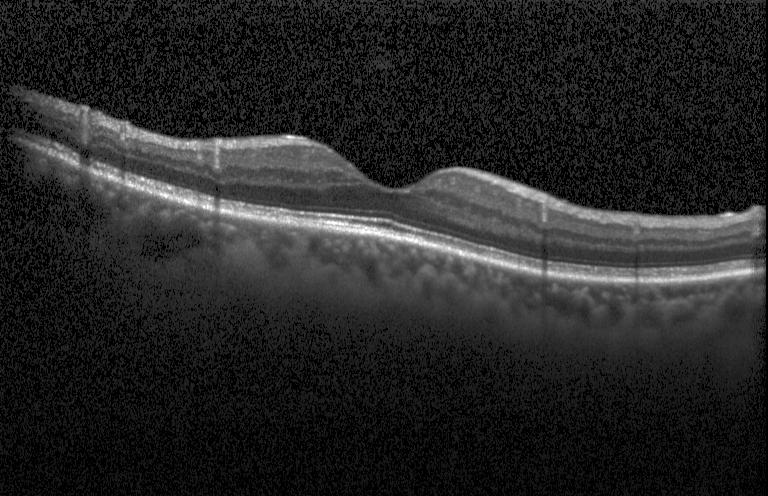 Horizontal scan through the fovea · spectral-domain optical coherence tomography · OCT B-scan · Heidelberg Spectralis. Impression: no choroidal neovascularization, diabetic macular edema, or drusen.